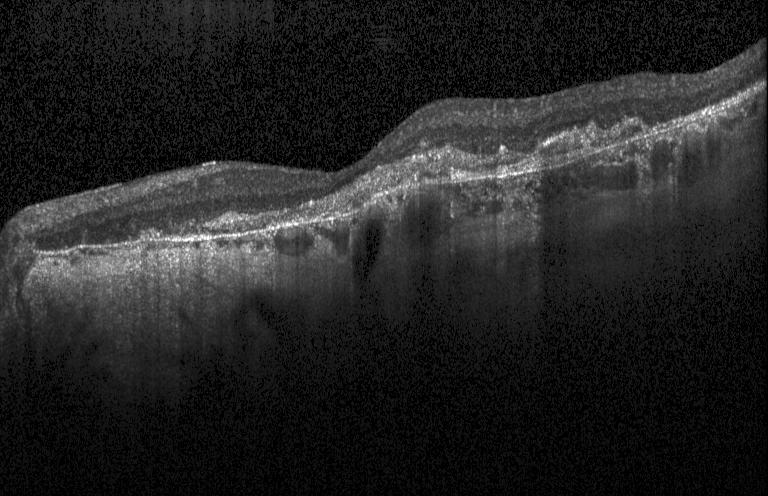

Diagnosis: choroidal neovascularization.